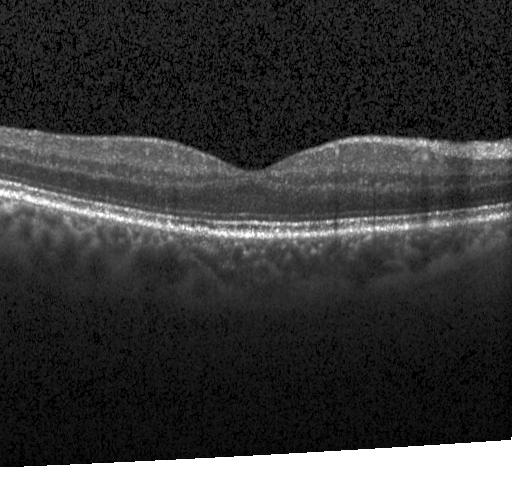

Optical coherence tomography scan
Finding: no CNV, no DME, and no drusen.